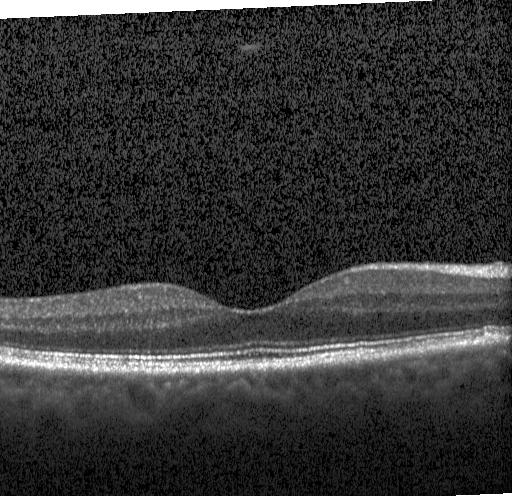
Retinal OCT B-scan.
No choroidal neovascularization, no diabetic macular edema, and no drusen.